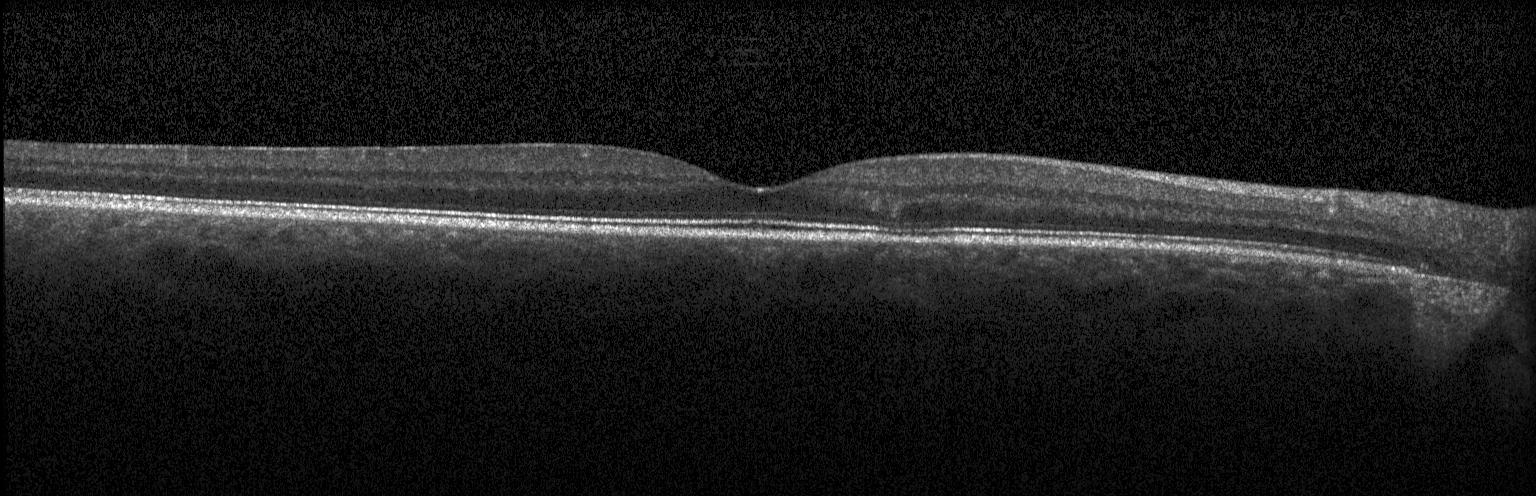 Fovea-centered. Spectral-domain OCT. Optical coherence tomography scan.
OCT finding: no choroidal neovascularization, diabetic macular edema, or drusen.